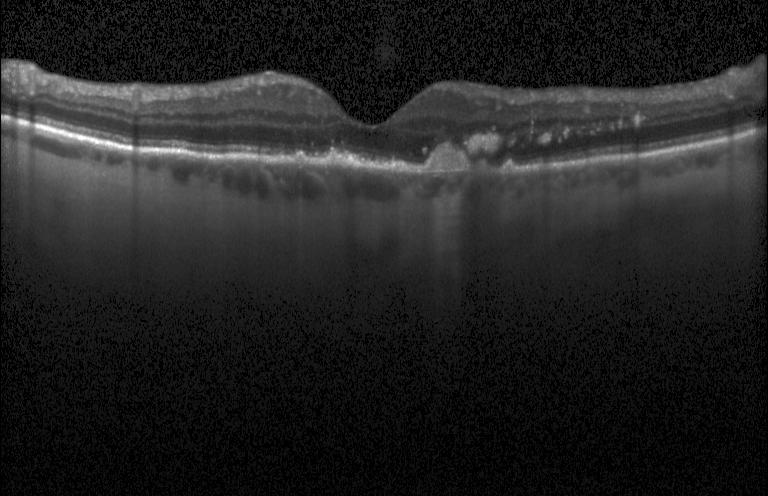

Optical coherence tomography scan, SD-OCT, through the macula, acquired on a Heidelberg Spectralis. Finding: drusen.